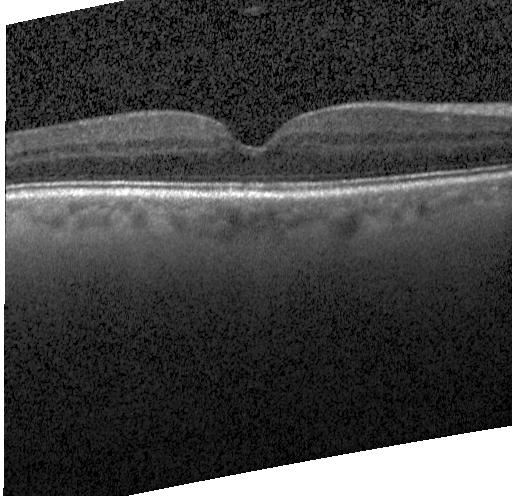
Optical coherence tomography B-scan.
The scan shows no choroidal neovascularization, diabetic macular edema, or drusen.